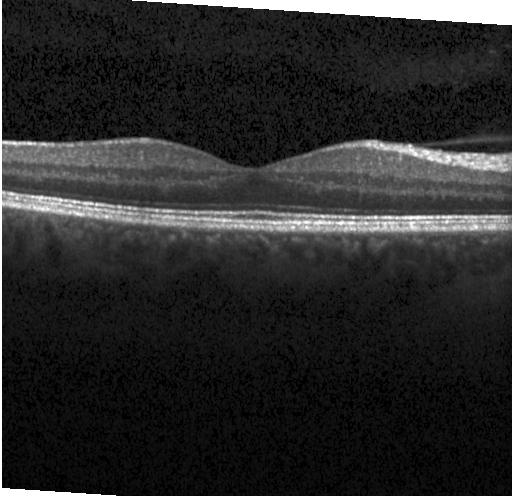
Finding: no CNV, no DME, and no drusen.